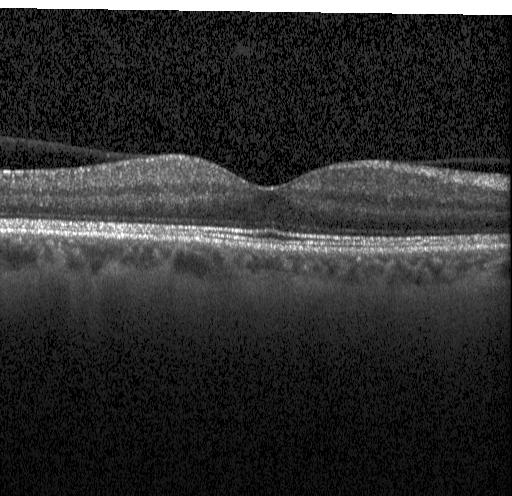 Spectral-domain OCT B-scan: no evidence of choroidal neovascularization, diabetic macular edema, or drusen.